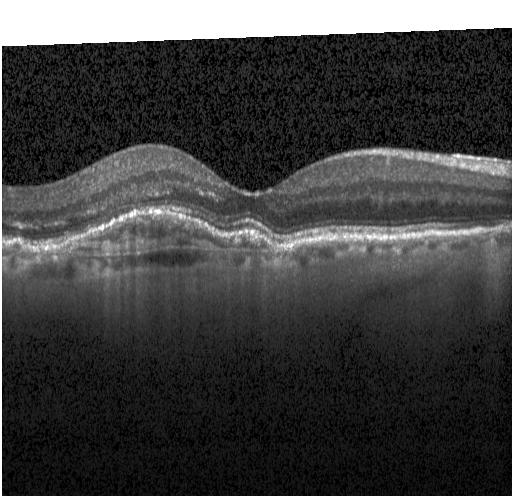

Acquired on a Heidelberg Spectralis · SD-OCT · OCT line scan — Dx: a choroidal neovascular membrane.